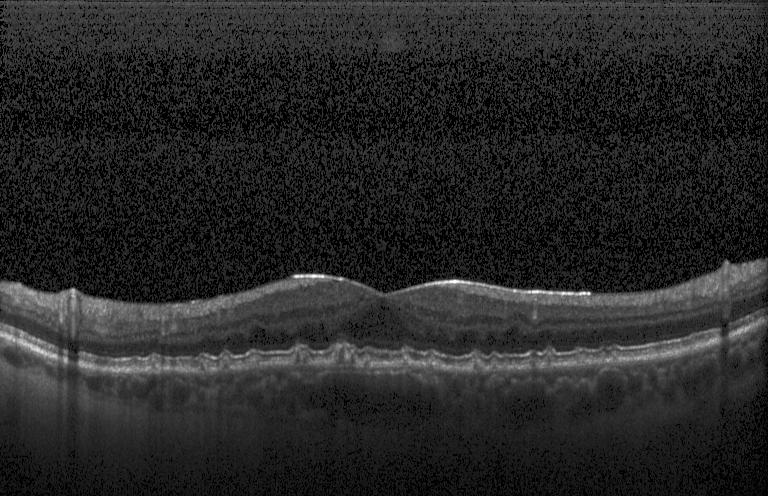
Assessment: sub-RPE drusenoid deposits.